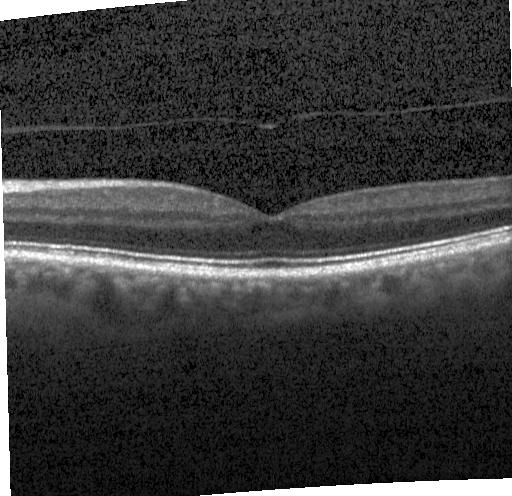
Through the macula. OCT B-scan. Instrument: Heidelberg Spectralis. SD-OCT — Diagnosis: no choroidal neovascularization, diabetic macular edema, or drusen.